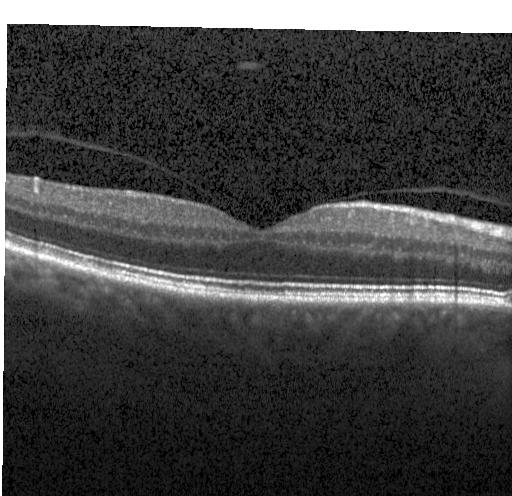
Horizontal scan through the fovea. Optical coherence tomography scan.
Diagnosis: no choroidal neovascularization, diabetic macular edema, or drusen.